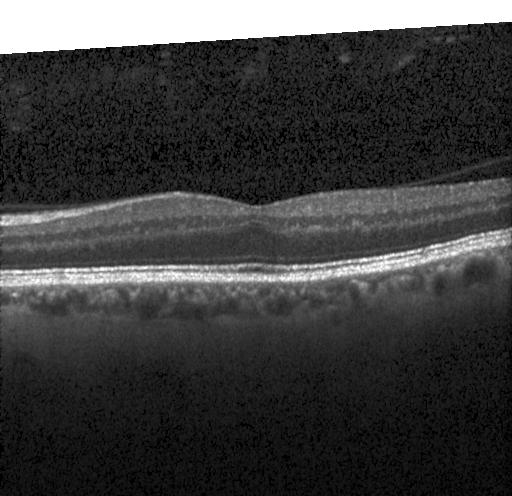

The scan shows no evidence of choroidal neovascularization, diabetic macular edema, or drusen.